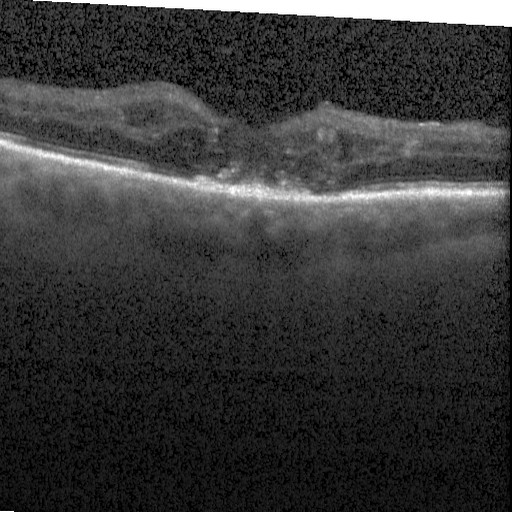

Dx: diabetic macular edema (DME).